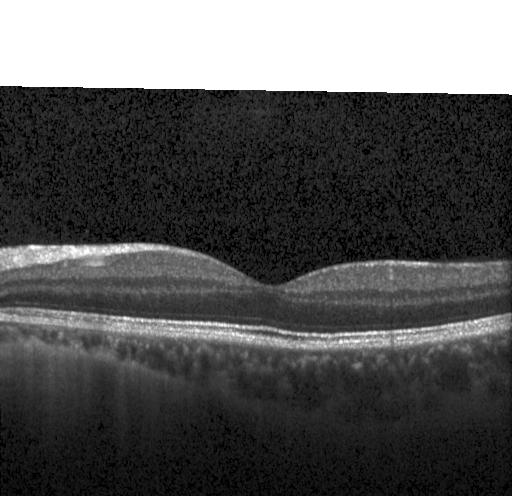

Optical coherence tomography scan, centered on the fovea, instrument: Heidelberg Spectralis — Impression: no evidence of CNV, DME, or drusen.